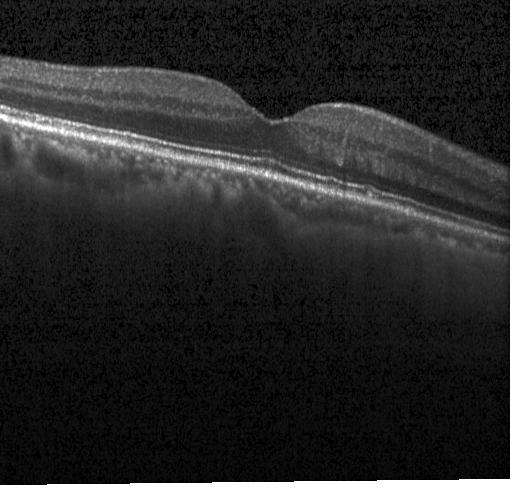 Heidelberg Spectralis · SD-OCT · through the macula · OCT B-scan.
Impression: no choroidal neovascularization, no diabetic macular edema, and no drusen.